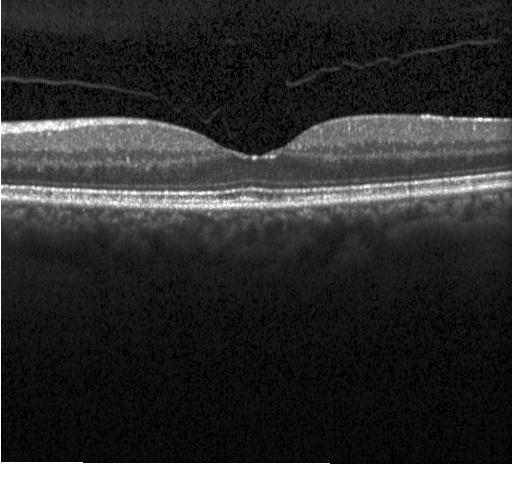
Optical coherence tomography B-scan. Heidelberg Spectralis. The scan shows no evidence of choroidal neovascularization, diabetic macular edema, or drusen.